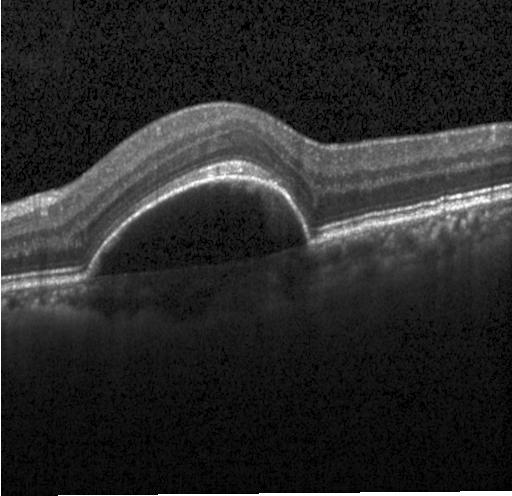 OCT B-scan; spectral-domain optical coherence tomography; instrument: Heidelberg Spectralis; fovea-centered.
Diagnosis: a choroidal neovascular membrane.